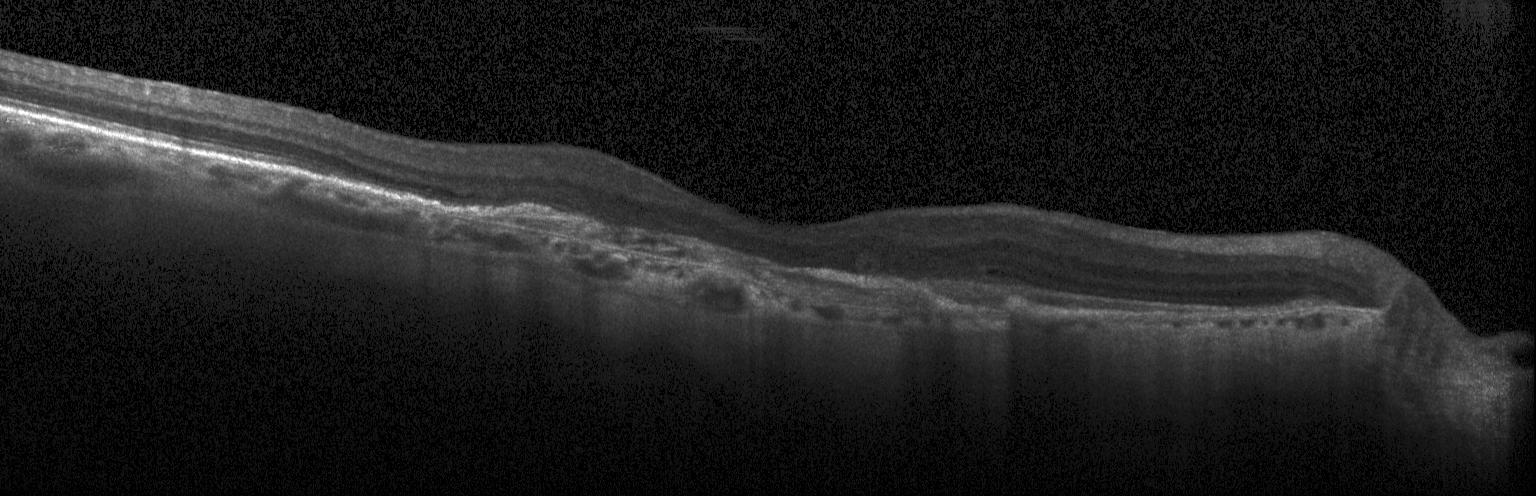

OCT line scan · through the macula · SD-OCT · acquired on a Heidelberg Spectralis
The scan shows choroidal neovascularization (CNV).